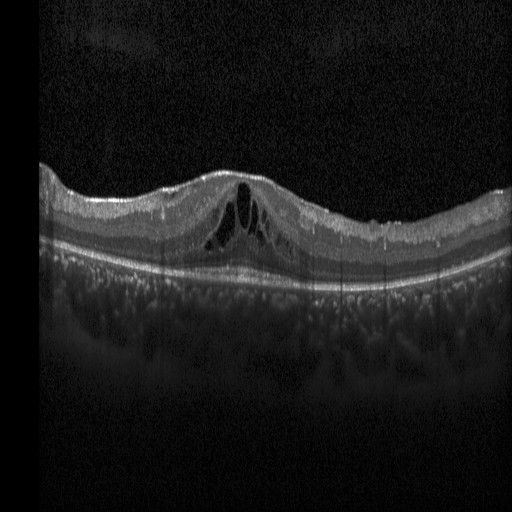
OCT B-scan. Dx: diabetic macular edema (DME).